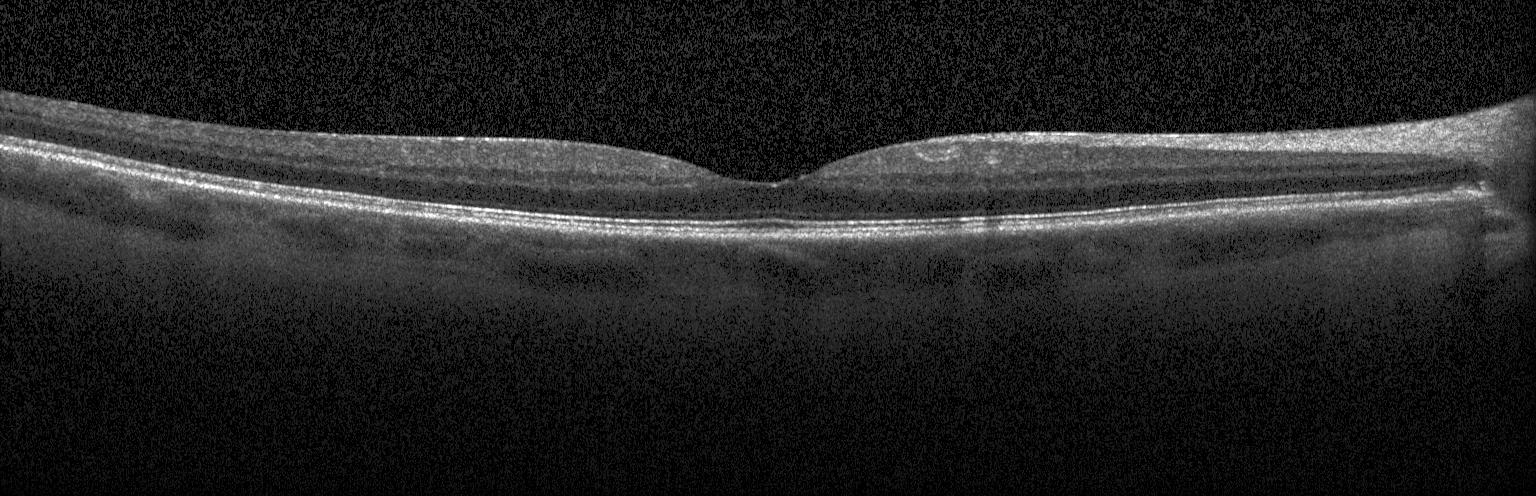 Macular OCT: no evidence of choroidal neovascularization, diabetic macular edema, or drusen.